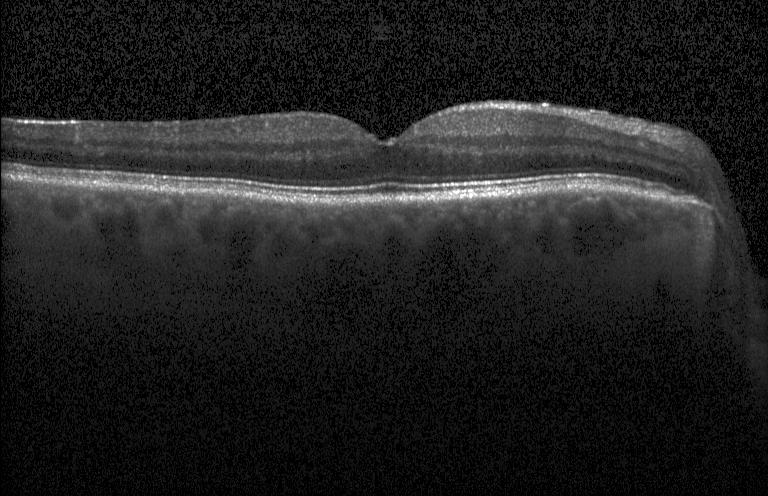 Retinal OCT B-scan. Macular scan. Diagnosis: neither choroidal neovascularization, diabetic macular edema, nor drusen.